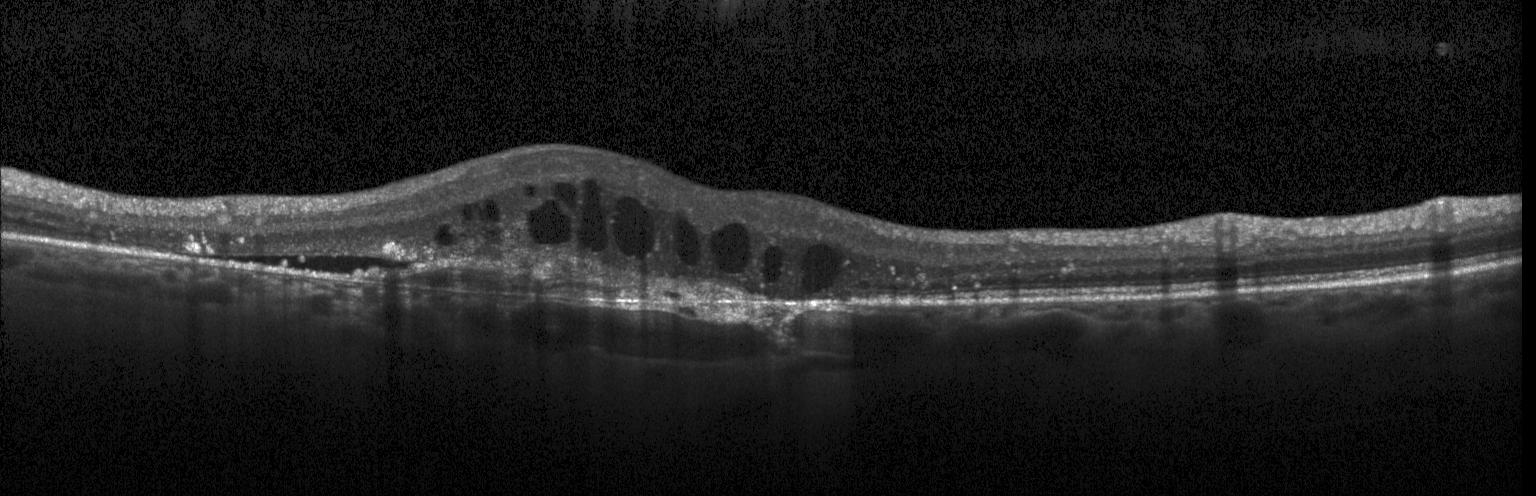
Centered on the fovea. Spectral-domain optical coherence tomography. OCT line scan. Heidelberg Spectralis OCT system.
OCT finding: choroidal neovascularization (CNV).